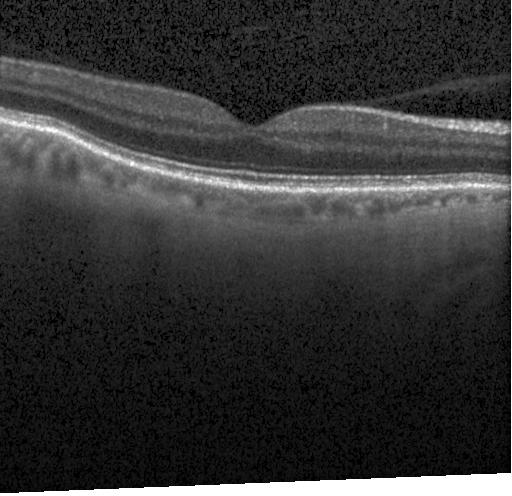 Retinal OCT cross-section — Diagnosis: no choroidal neovascularization, no diabetic macular edema, and no drusen.